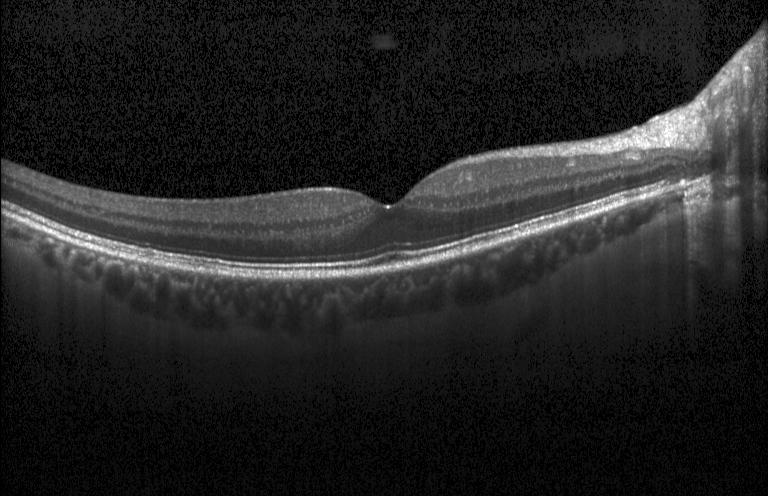
Horizontal scan through the fovea; optical coherence tomography B-scan; Heidelberg Spectralis. This B-scan demonstrates neither choroidal neovascularization, diabetic macular edema, nor drusen.